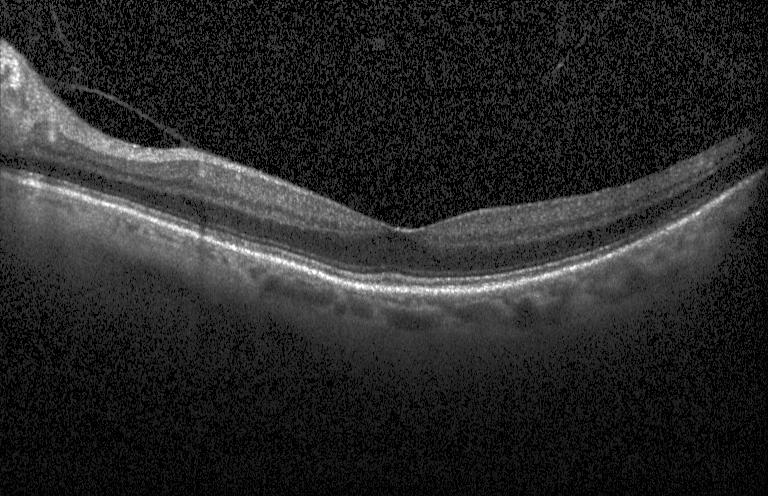

OCT B-scan, through the macula, Heidelberg Spectralis OCT system. Diagnosis: no choroidal neovascularization, diabetic macular edema, or drusen.